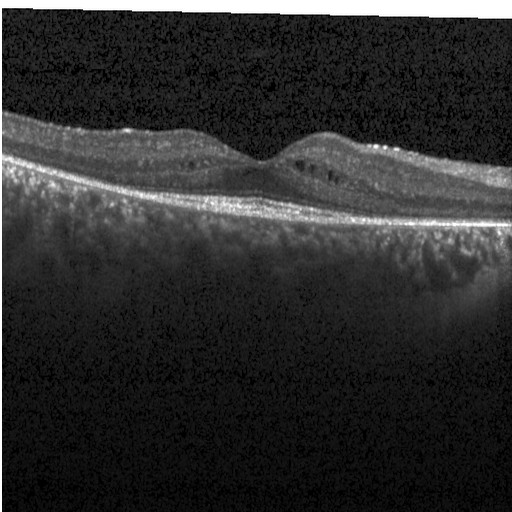

Finding: DME.